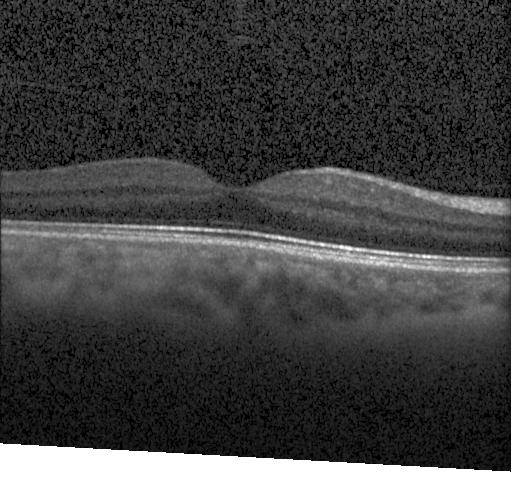 Macular OCT: no choroidal neovascularization, diabetic macular edema, or drusen.